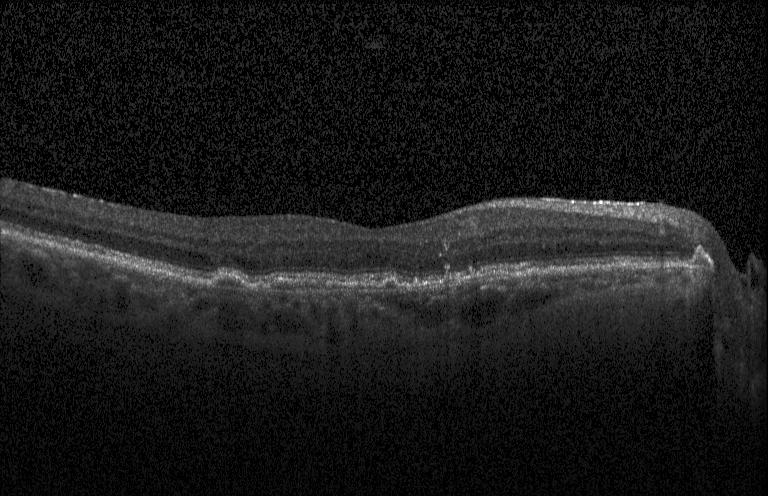 Retinal OCT cross-section.
Diagnosis: CNV.